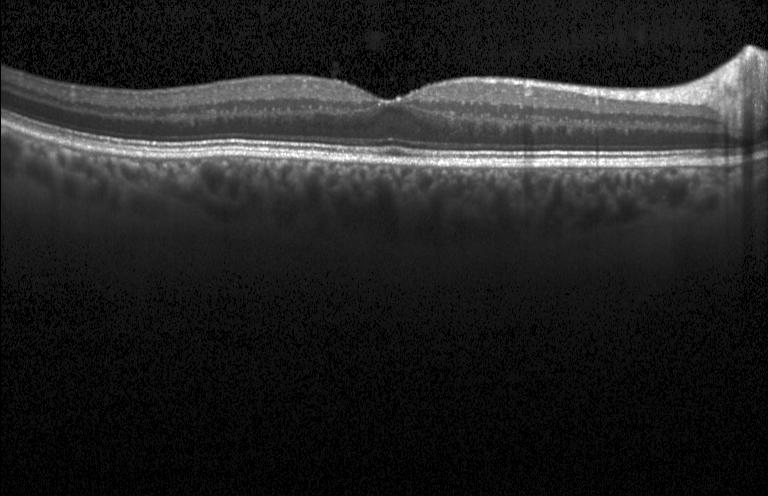 OCT B-scan showing no evidence of choroidal neovascularization, diabetic macular edema, or drusen.